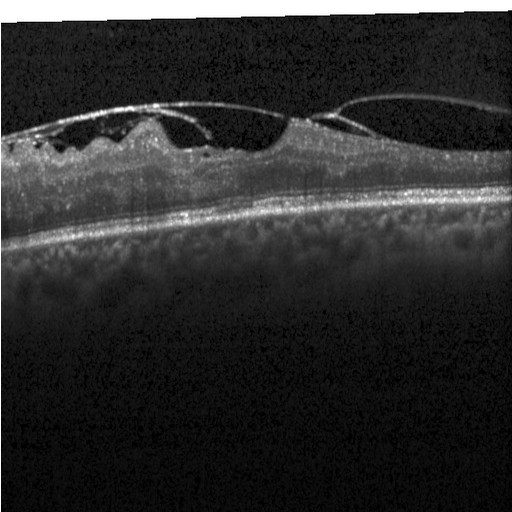

Impression: diabetic macular edema (DME).